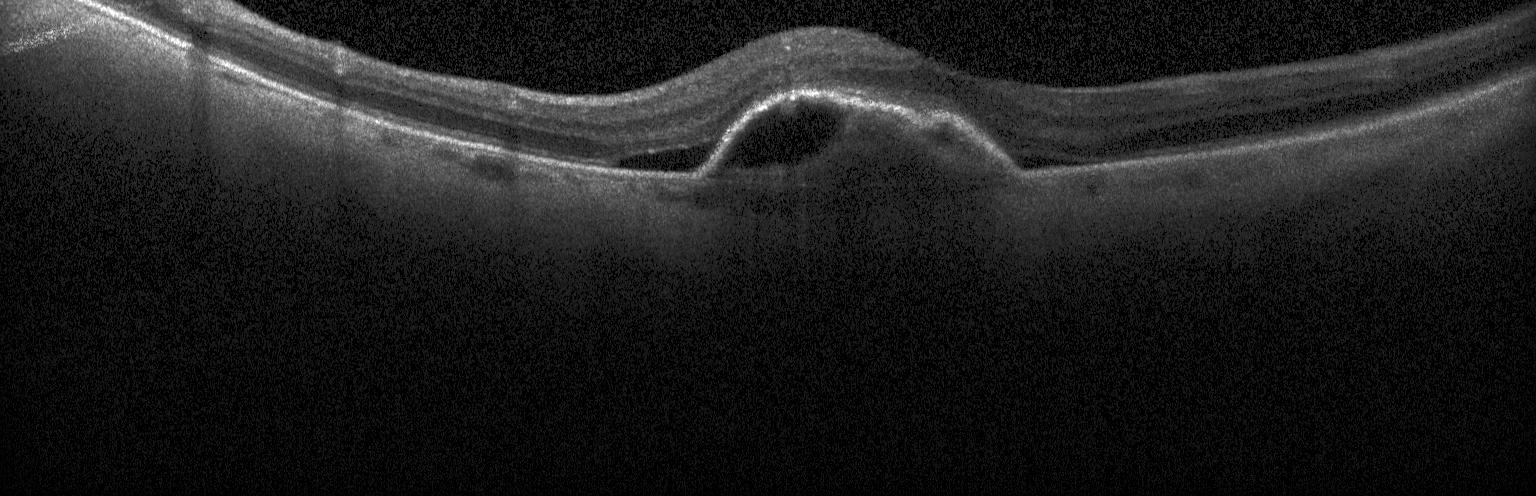

Fovea-centered; optical coherence tomography B-scan; Heidelberg Spectralis OCT system.
OCT finding: choroidal neovascularization (CNV).